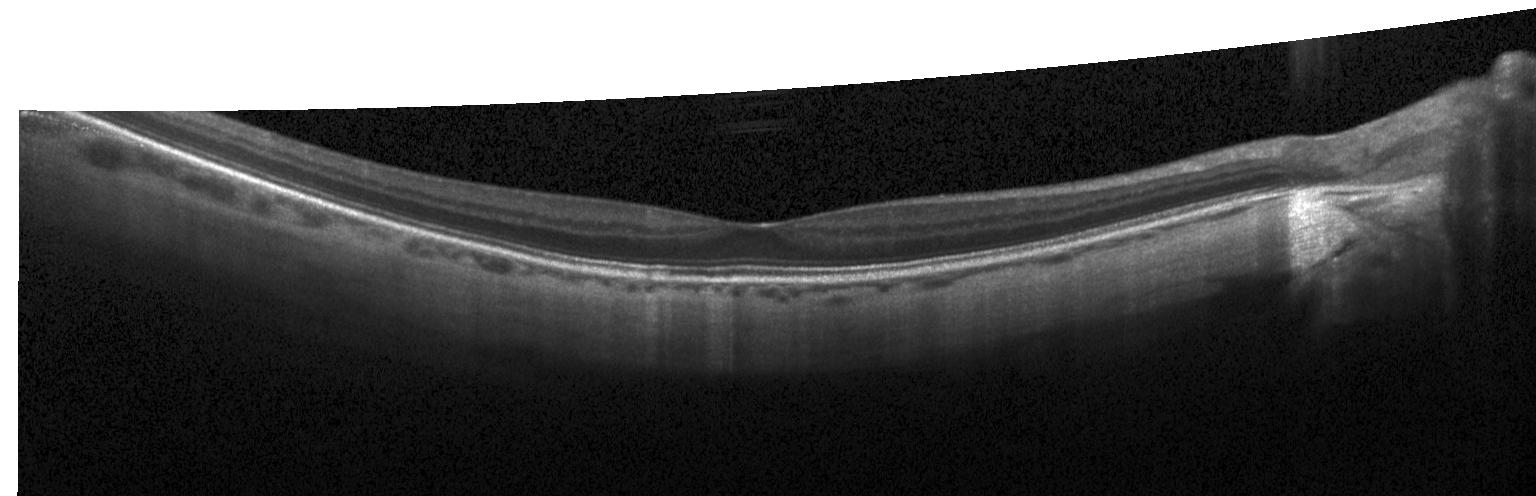 Optical coherence tomography B-scan · macular scan · Heidelberg Spectralis.
Macular OCT: neither choroidal neovascularization, diabetic macular edema, nor drusen.